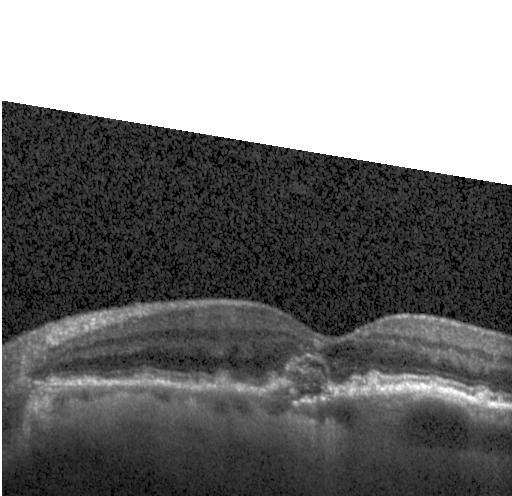

Macular OCT: a choroidal neovascular membrane.